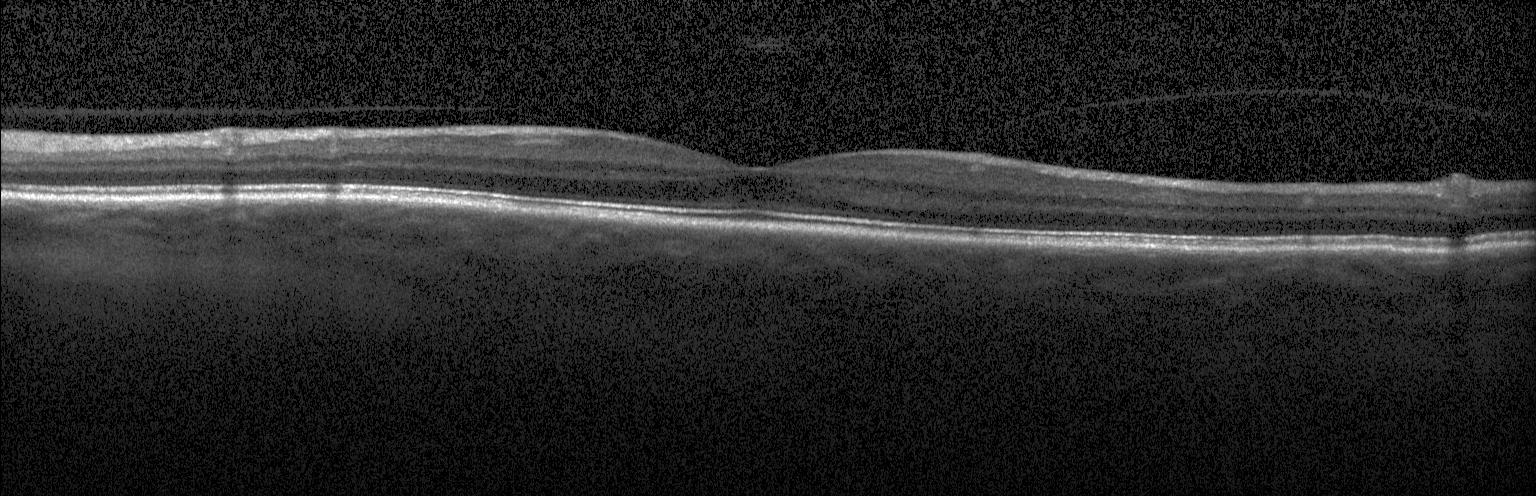

Assessment: no CNV, DME, or drusen.